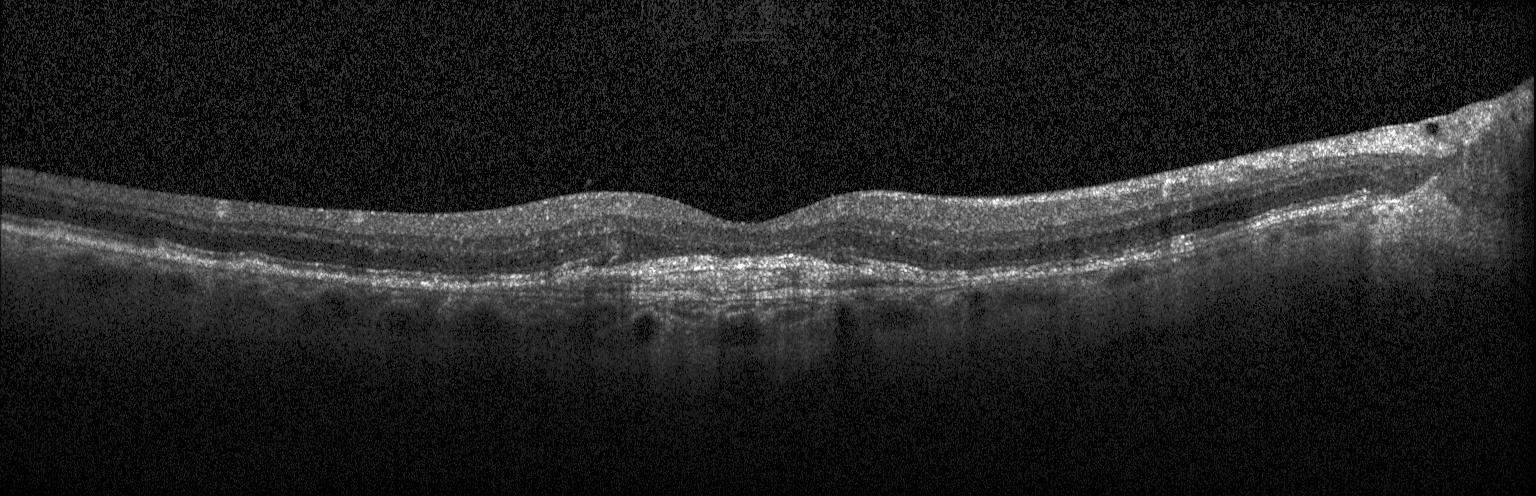 Macular scan. Optical coherence tomography B-scan. Impression: a choroidal neovascular membrane.